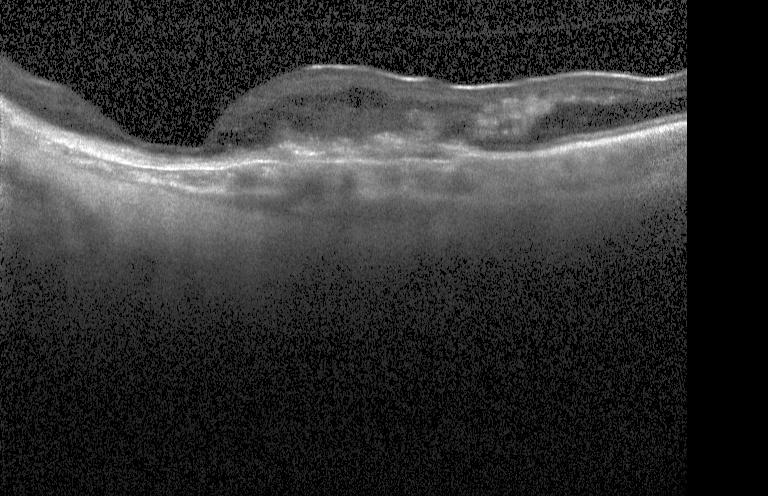

Macular OCT demonstrating a choroidal neovascular membrane.